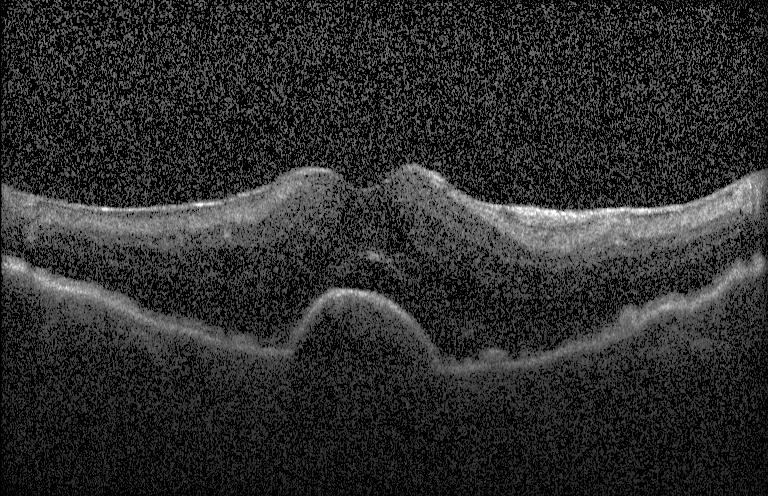

Assessment: choroidal neovascularization.